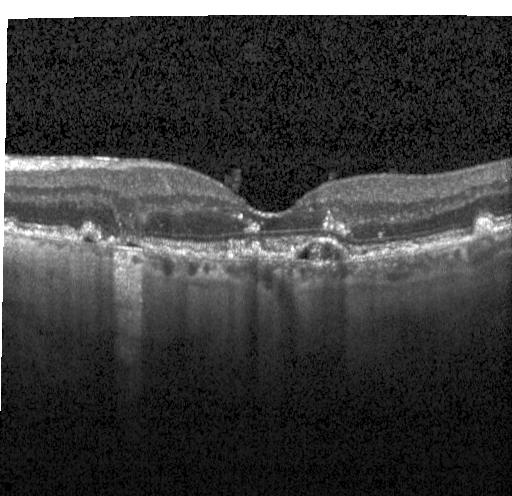 Heidelberg Spectralis OCT system · optical coherence tomography B-scan. Dx: CNV.